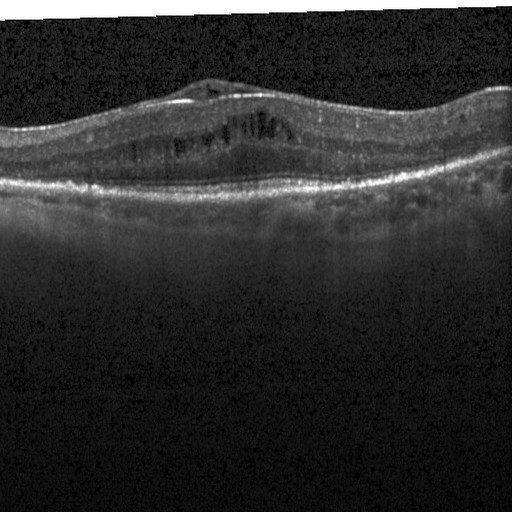 Spectral-domain optical coherence tomography; optical coherence tomography scan; horizontal scan through the fovea
Diagnosis: diabetic macular edema.